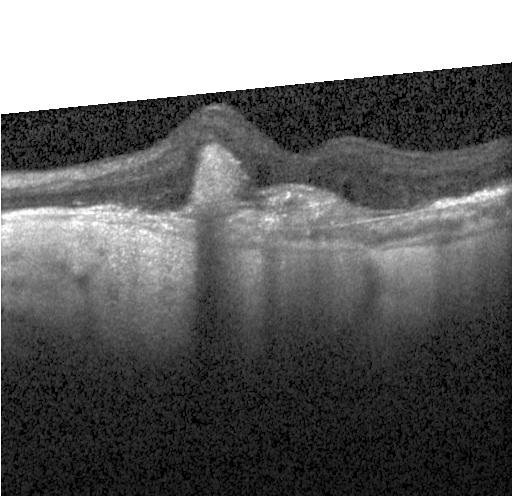

Retinal OCT B-scan.
Impression: a choroidal neovascular membrane.